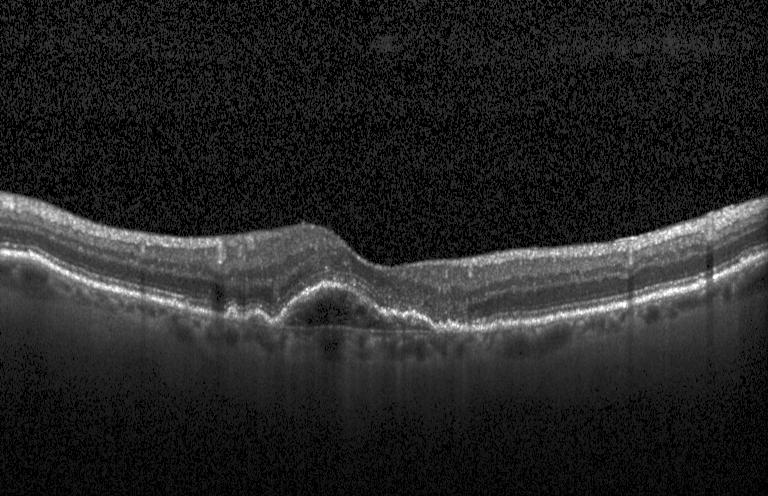 Heidelberg Spectralis OCT system, optical coherence tomography scan, fovea-centered.
Diagnosis: choroidal neovascularization (CNV).